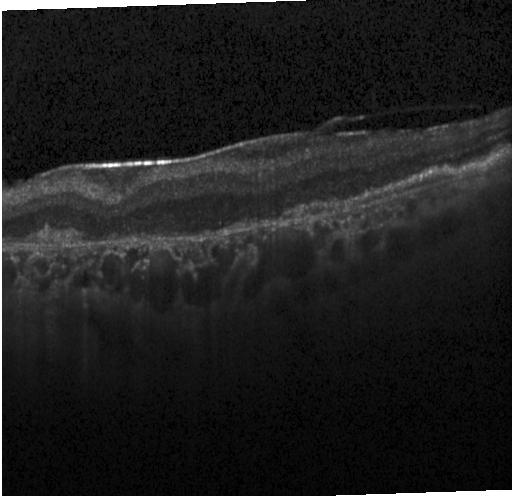 SD-OCT. Macular scan. Instrument: Heidelberg Spectralis. Retinal OCT cross-section — Impression: choroidal neovascularization (CNV).